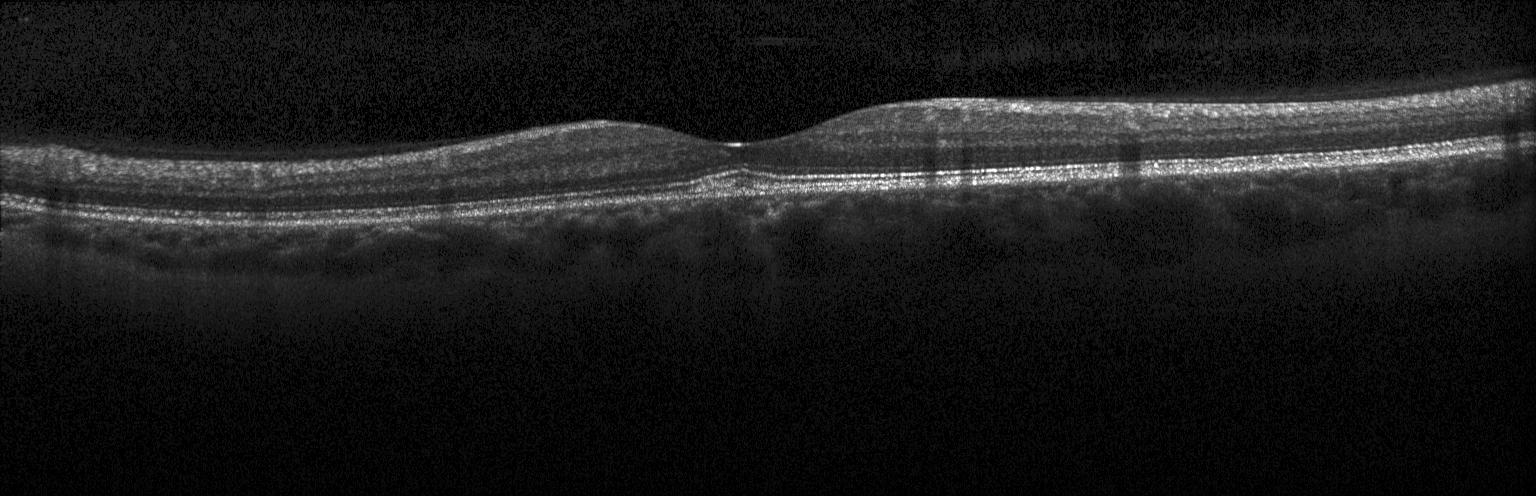 This B-scan demonstrates no CNV, no DME, and no drusen.